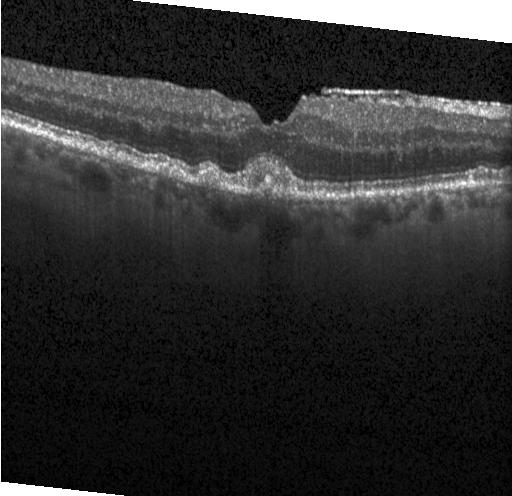

Optical coherence tomography B-scan · fovea-centered.
Impression: drusen.